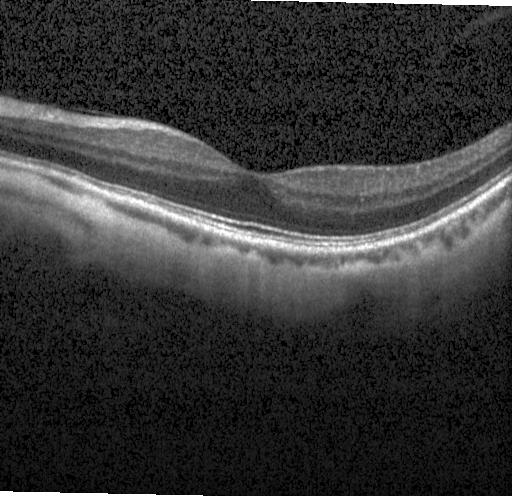 Retinal OCT B-scan. Assessment: no evidence of choroidal neovascularization, diabetic macular edema, or drusen.